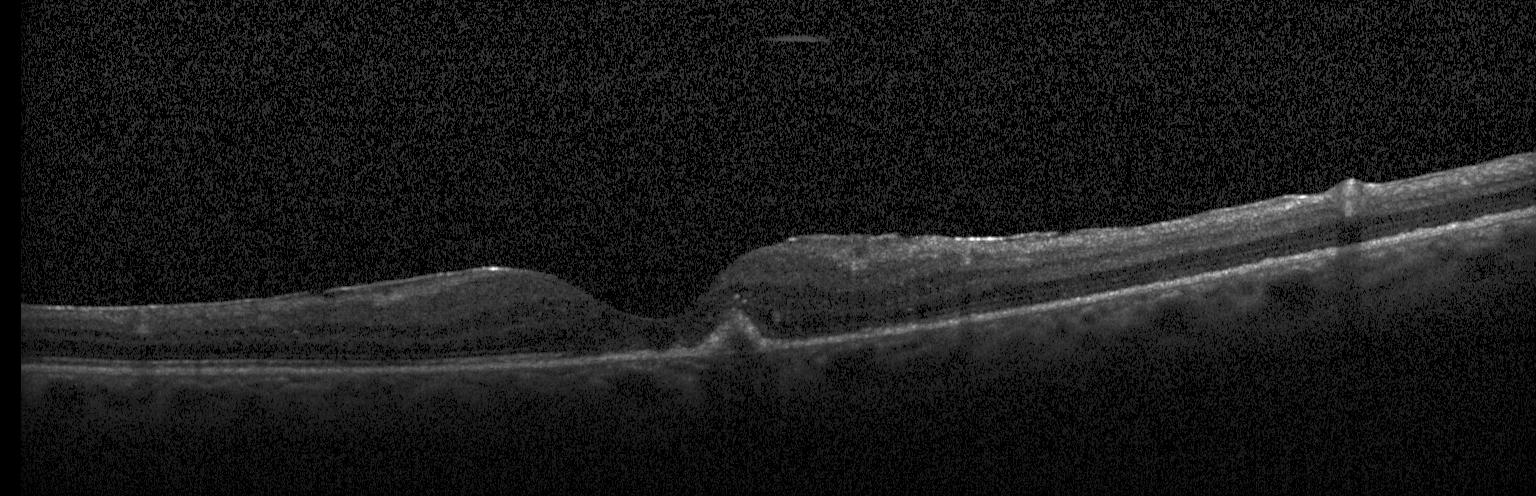

Acquired on a Heidelberg Spectralis. Retinal OCT B-scan. Centered on the fovea
Diagnosis: a choroidal neovascular membrane.